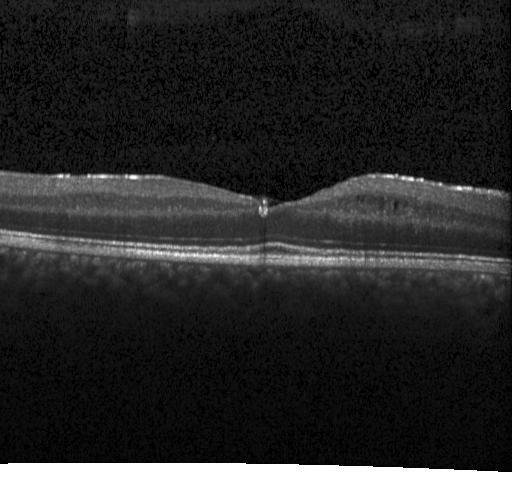 Retinal OCT B-scan; Heidelberg Spectralis OCT system; spectral-domain optical coherence tomography.
Macular OCT: diabetic macular edema (DME).